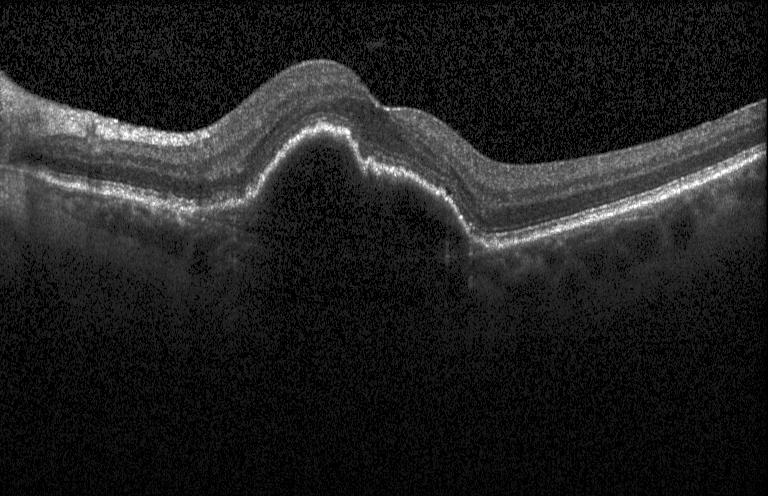
Spectral-domain OCT B-scan: choroidal neovascularization (CNV).